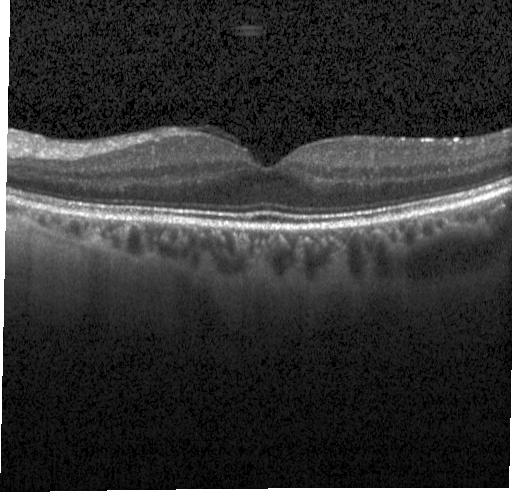
Impression: no CNV, no DME, and no drusen.